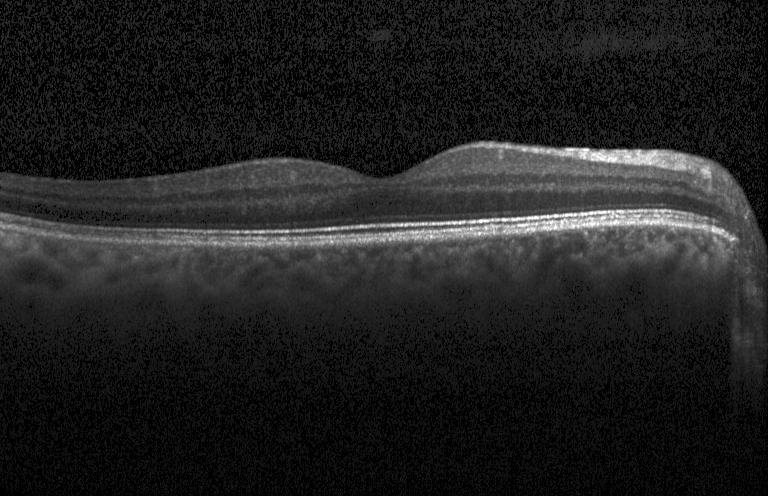

Retinal OCT cross-section showing neither CNV, DME, nor drusen.